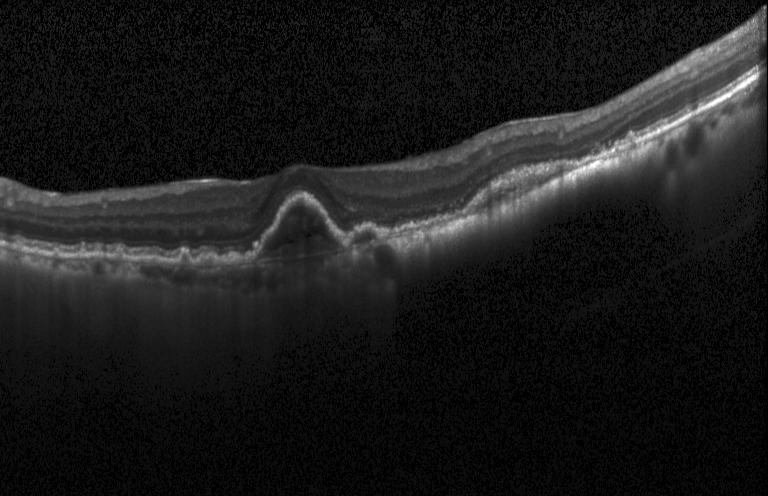
This B-scan demonstrates a choroidal neovascular membrane.